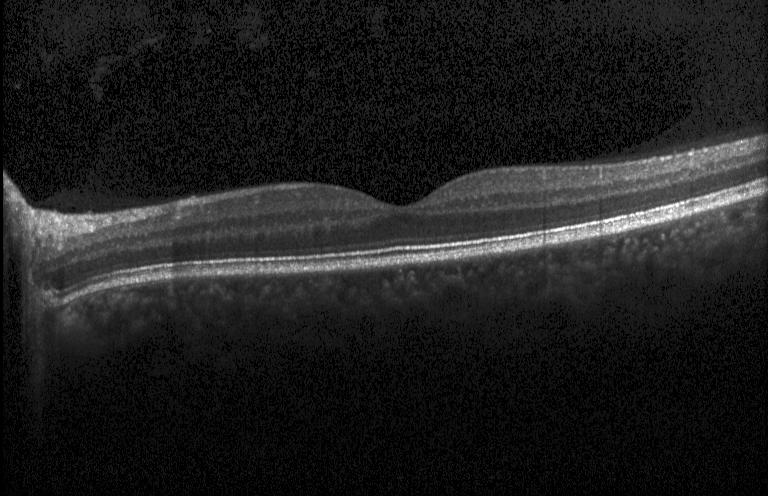
Macular OCT demonstrating neither choroidal neovascularization, diabetic macular edema, nor drusen.